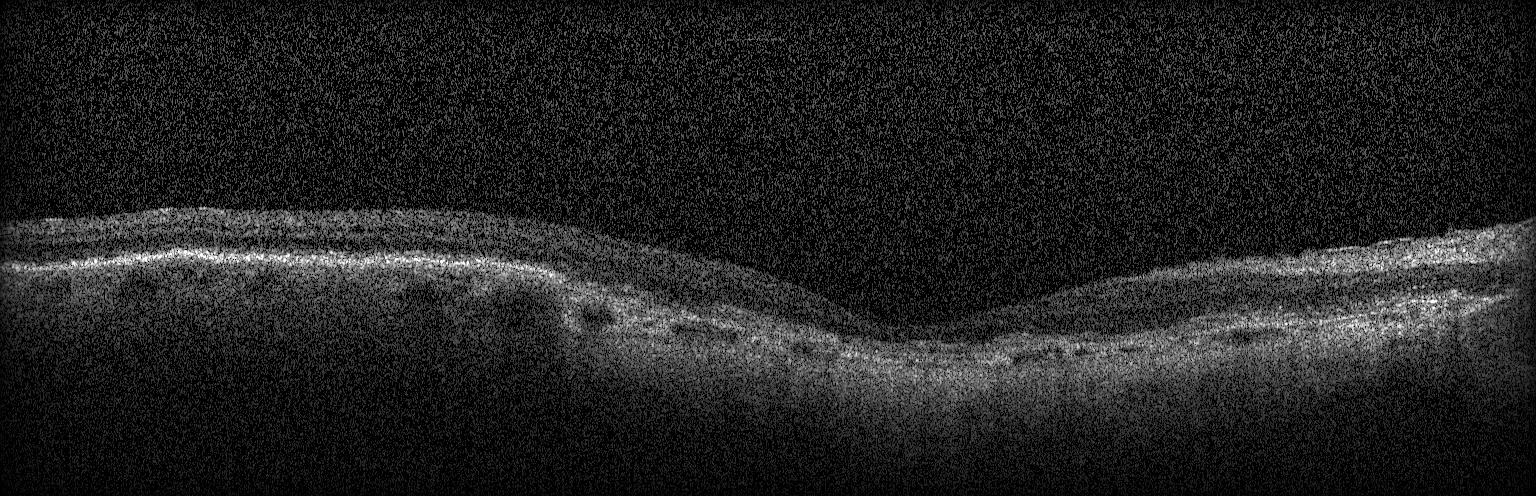 Finding: a choroidal neovascular membrane.